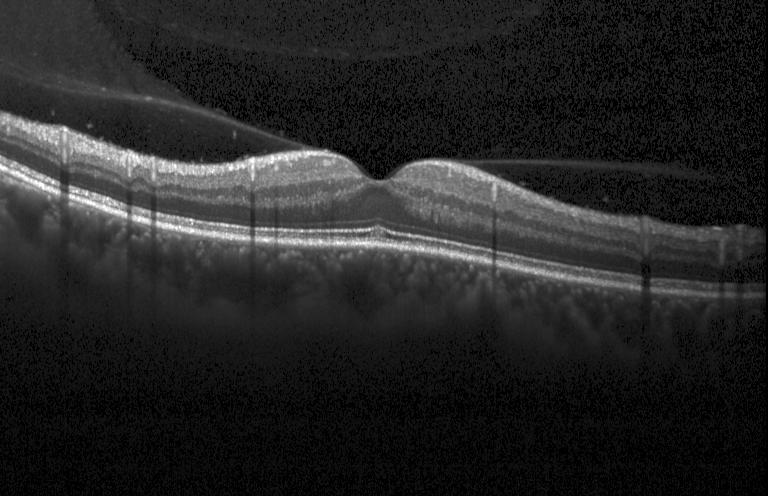

Retinal OCT cross-section. Spectral-domain optical coherence tomography. Horizontal scan through the fovea.
Impression: no CNV, no DME, and no drusen.